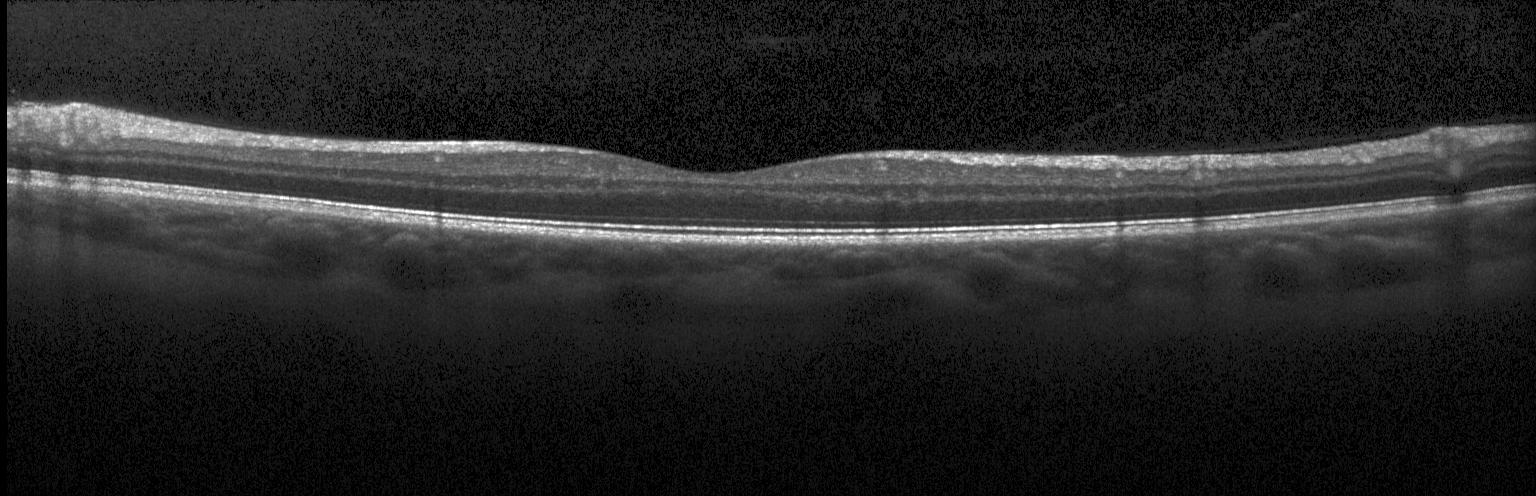

Optical coherence tomography scan, spectral-domain optical coherence tomography — Diagnosis: neither CNV, DME, nor drusen.